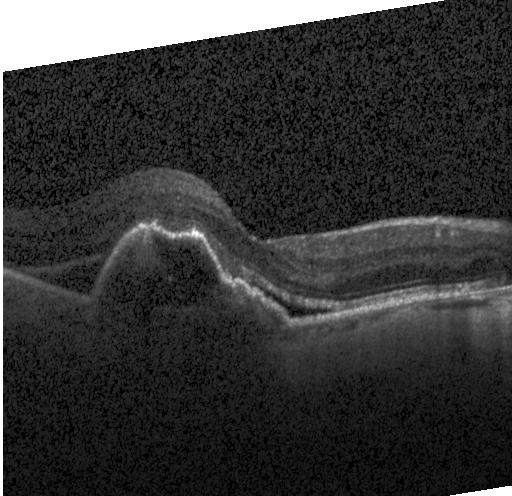
Optical coherence tomography scan. Horizontal scan through the fovea. Assessment: choroidal neovascularization.